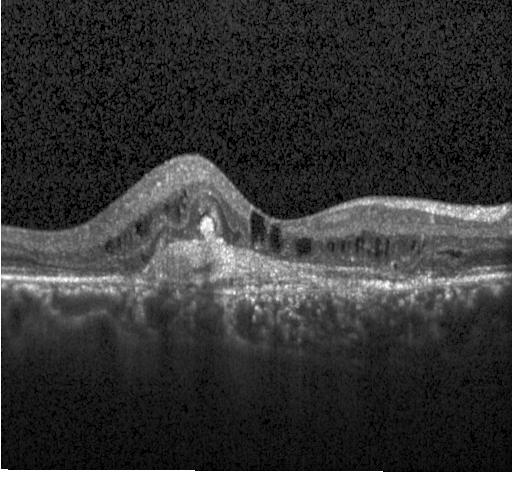
Retinal OCT cross-section — Assessment: choroidal neovascularization.